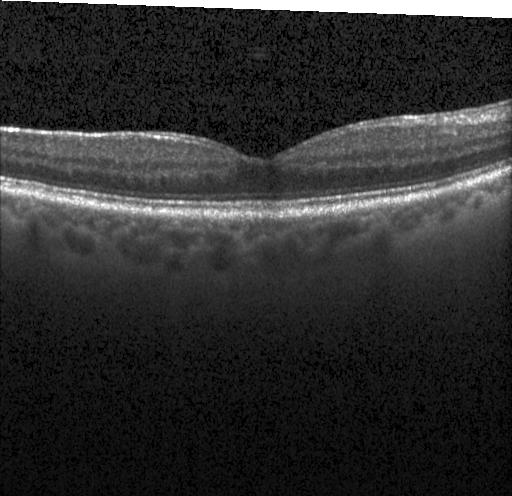 Finding: no CNV, DME, or drusen.